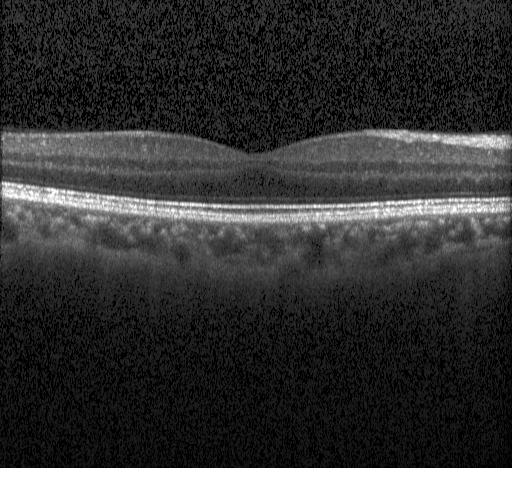 No evidence of choroidal neovascularization, diabetic macular edema, or drusen.